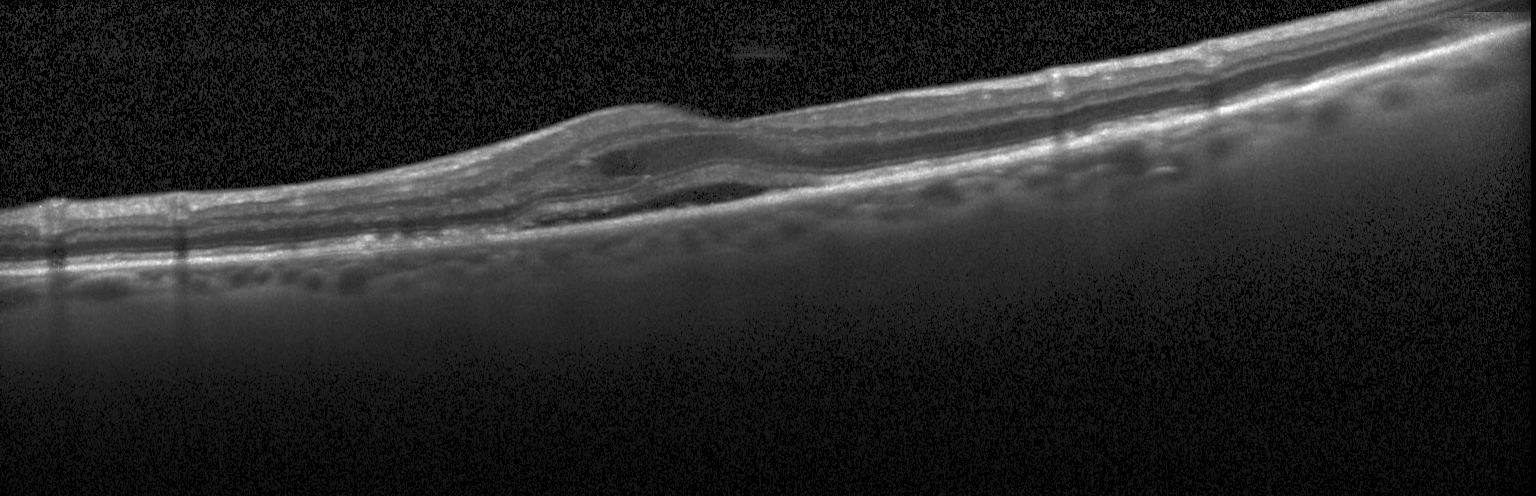

Retinal OCT B-scan. Finding: a choroidal neovascular membrane.